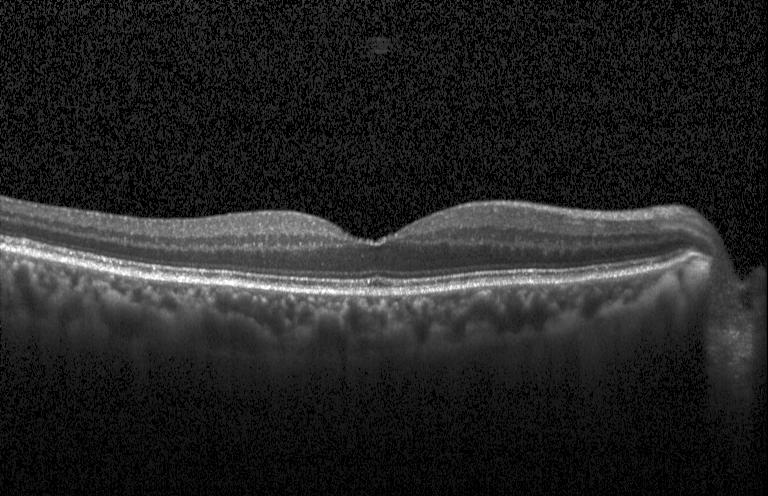

Retinal OCT B-scan — Dx: no evidence of choroidal neovascularization, diabetic macular edema, or drusen.